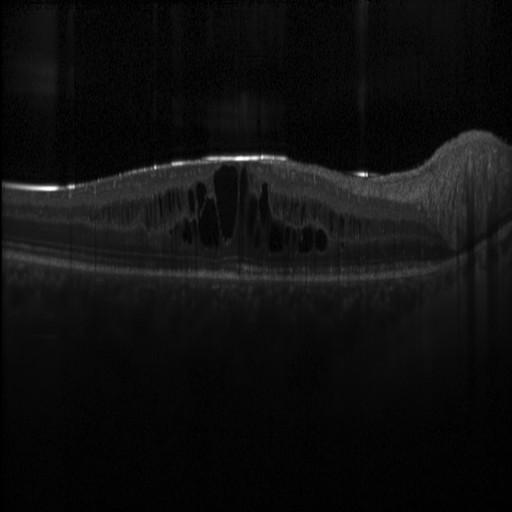

Optical coherence tomography B-scan. Spectral-domain OCT — This B-scan demonstrates DME.